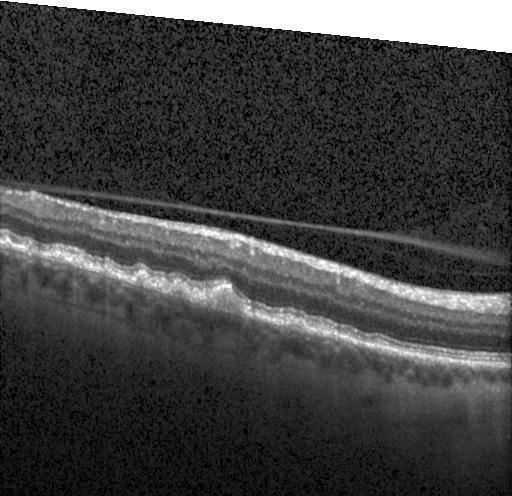 Optical coherence tomography B-scan, macular scan, instrument: Heidelberg Spectralis, SD-OCT
The scan shows sub-RPE drusenoid deposits.